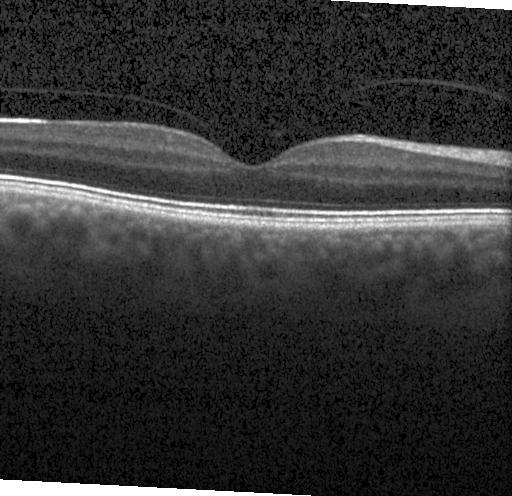
Macular scan. OCT line scan. Heidelberg Spectralis OCT system
The scan shows neither choroidal neovascularization, diabetic macular edema, nor drusen.